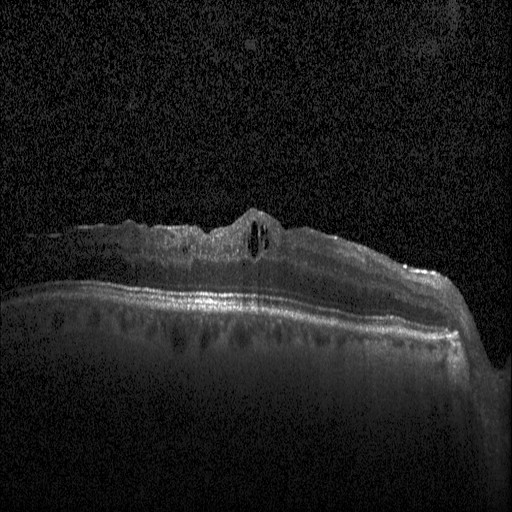
The scan shows diabetic macular edema.